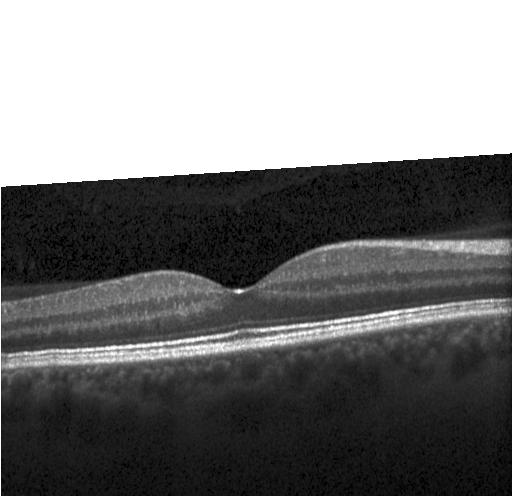 Diagnosis: no choroidal neovascularization, no diabetic macular edema, and no drusen.